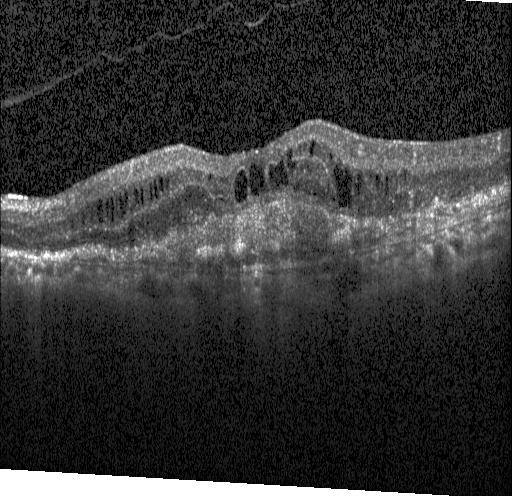 Spectral-domain OCT; Heidelberg Spectralis; through the macula; optical coherence tomography B-scan.
Assessment: a choroidal neovascular membrane.